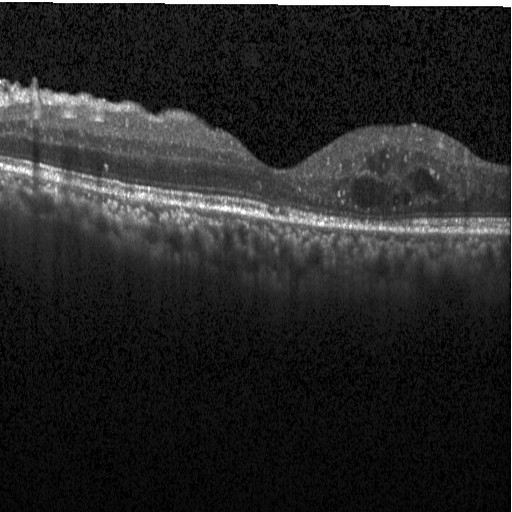
Heidelberg Spectralis · OCT B-scan · SD-OCT — Finding: diabetic macular edema.